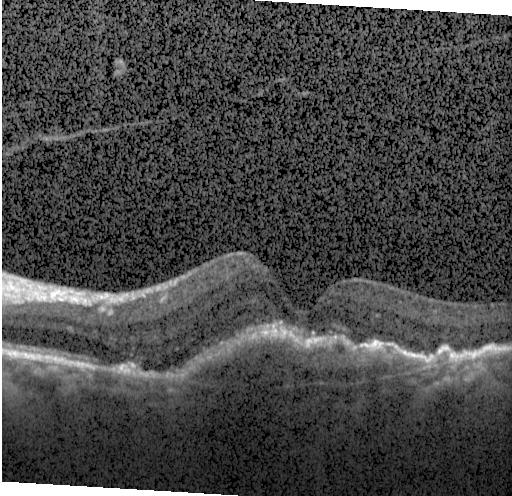
Finding: a choroidal neovascular membrane.